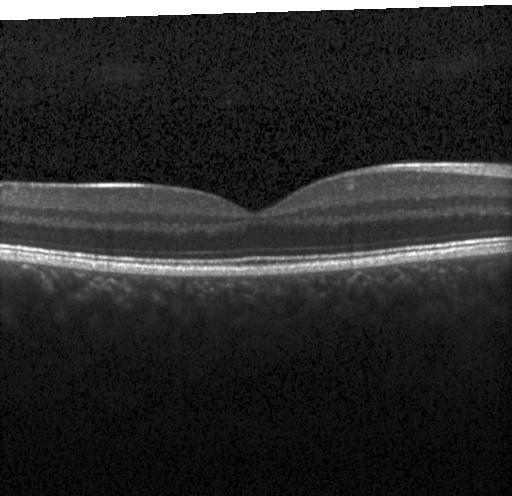
Heidelberg Spectralis, spectral-domain optical coherence tomography, retinal OCT B-scan, macular scan — Assessment: no CNV, no DME, and no drusen.